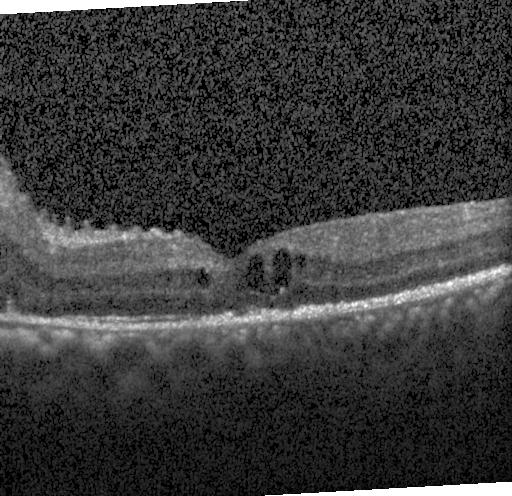

OCT B-scan; Heidelberg Spectralis OCT system; spectral-domain optical coherence tomography — The scan shows diabetic macular edema.